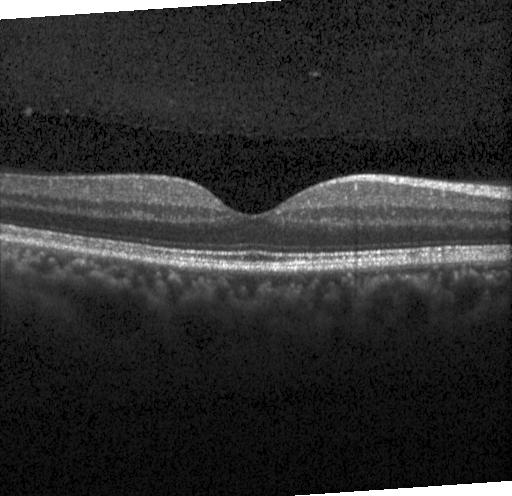
The scan shows no evidence of choroidal neovascularization, diabetic macular edema, or drusen.